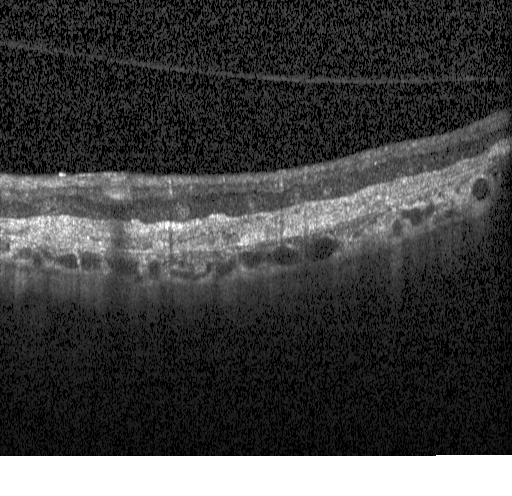

OCT line scan. Heidelberg Spectralis OCT system.
Diagnosis: choroidal neovascularization (CNV).